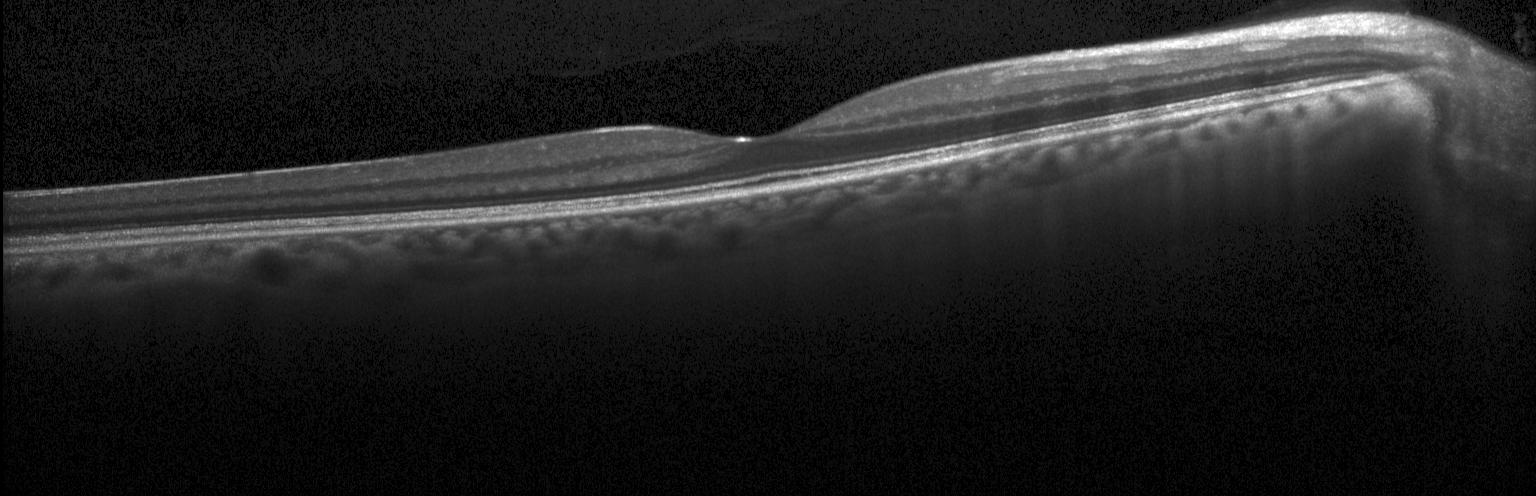 Optical coherence tomography B-scan. SD-OCT — Impression: no evidence of choroidal neovascularization, diabetic macular edema, or drusen.